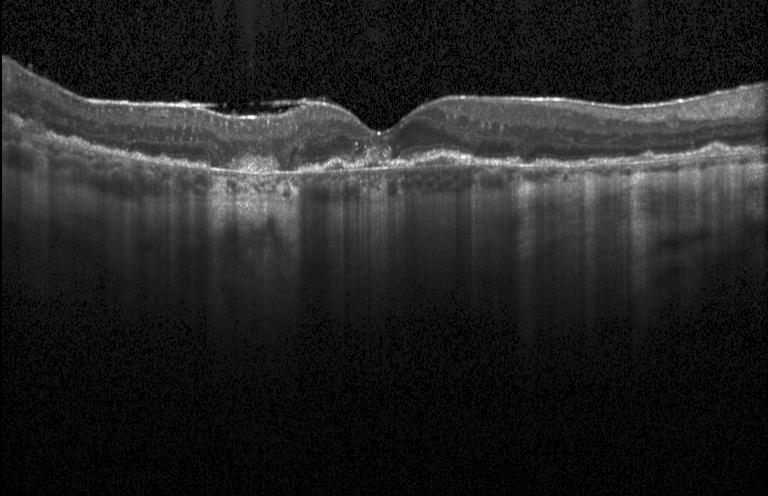 Spectral-domain OCT. Optical coherence tomography B-scan. Macular scan. Heidelberg Spectralis OCT system. Finding: choroidal neovascularization.